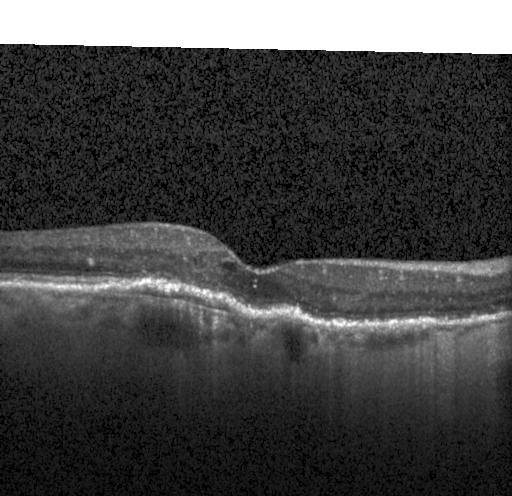
Spectral-domain optical coherence tomography; centered on the fovea; OCT B-scan; Heidelberg Spectralis.
Impression: a choroidal neovascular membrane.